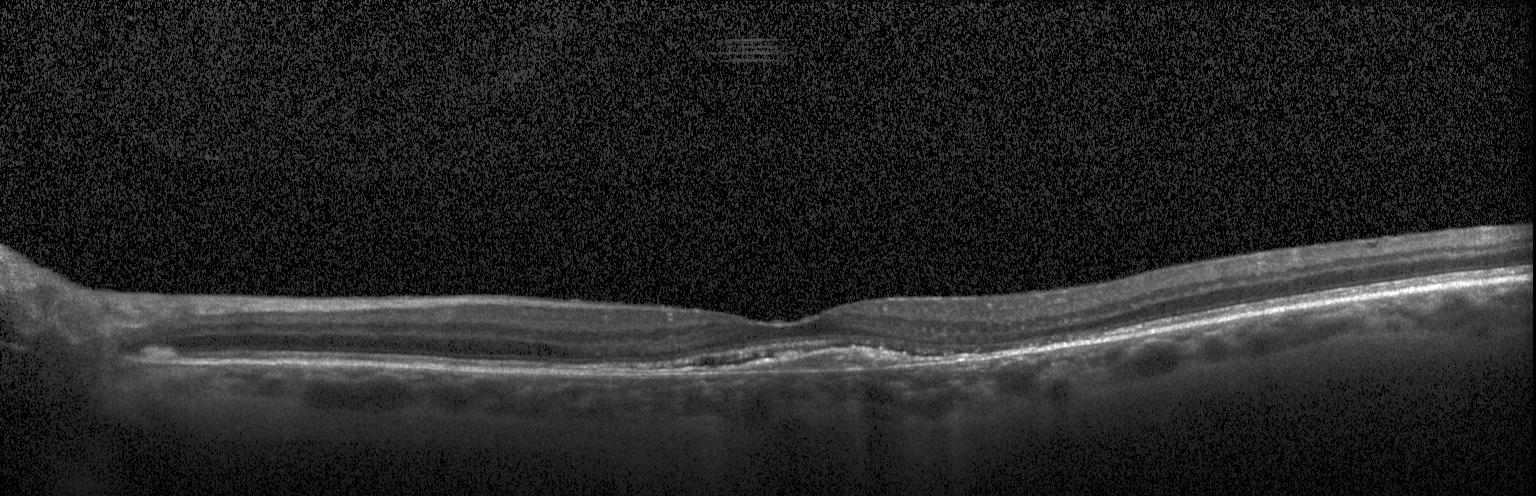

Finding: choroidal neovascularization.